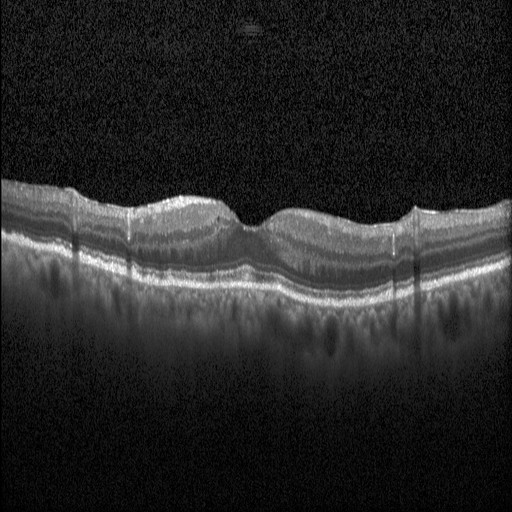 Retinal OCT B-scan.
DME.